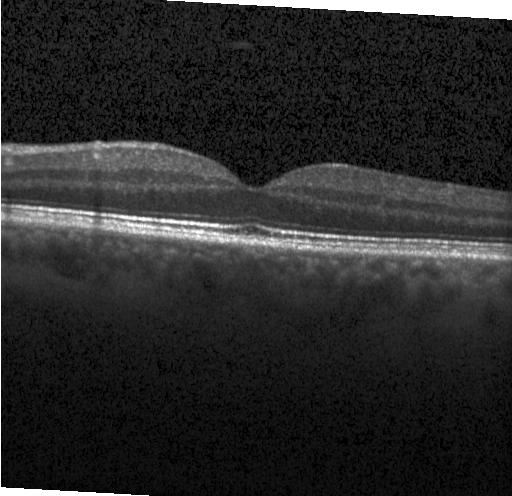
OCT B-scan — OCT finding: no CNV, no DME, and no drusen.